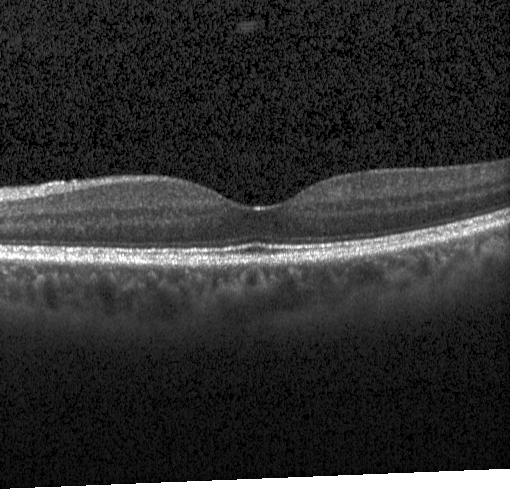

Finding: no choroidal neovascularization, diabetic macular edema, or drusen.